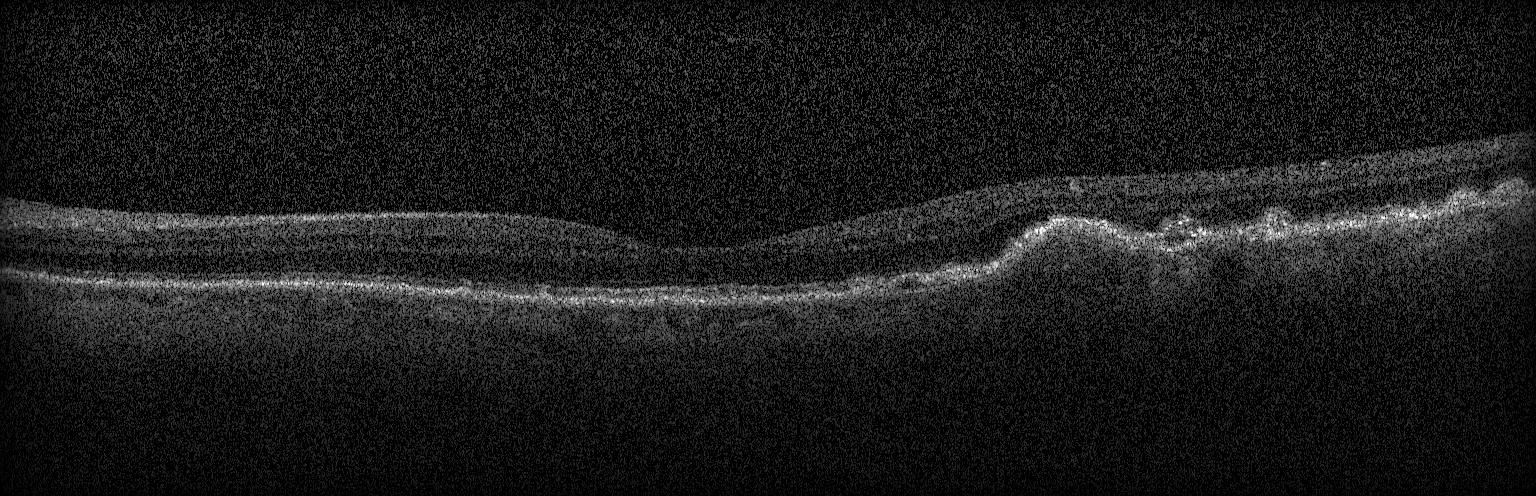
Diagnosis: CNV.